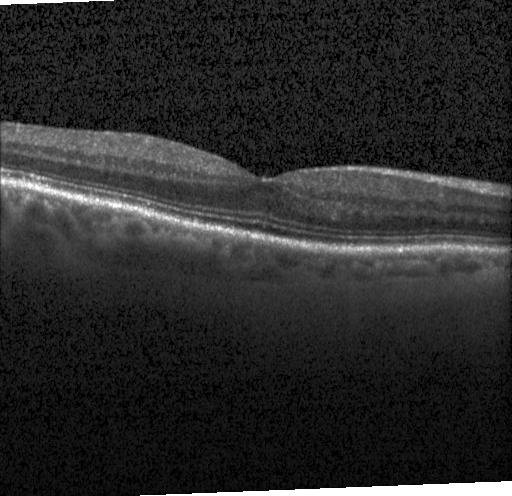 Spectral-domain optical coherence tomography, instrument: Heidelberg Spectralis, retinal OCT B-scan
Macular OCT: no evidence of CNV, DME, or drusen.